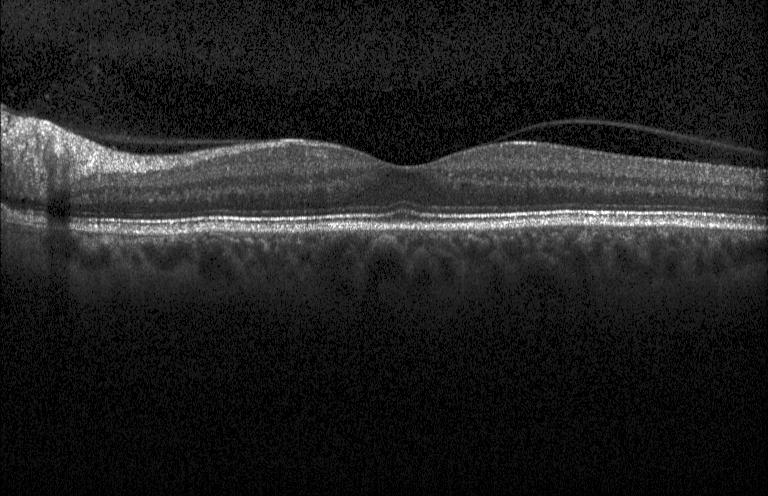 Diagnosis: neither CNV, DME, nor drusen.